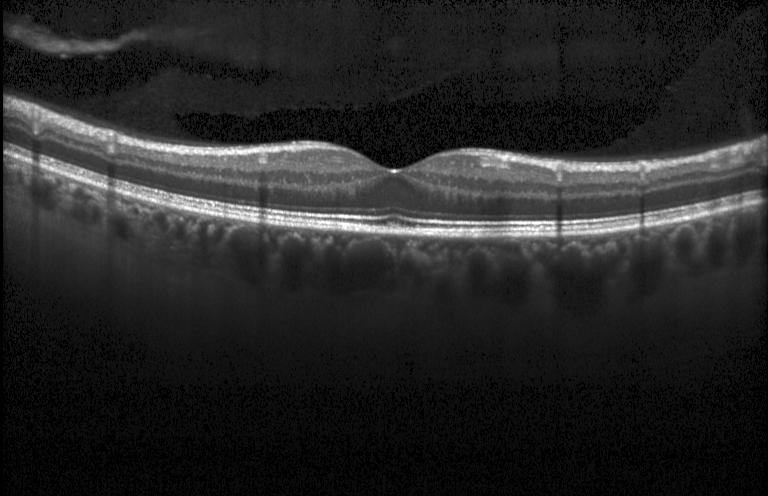 OCT B-scan.
Impression: neither choroidal neovascularization, diabetic macular edema, nor drusen.